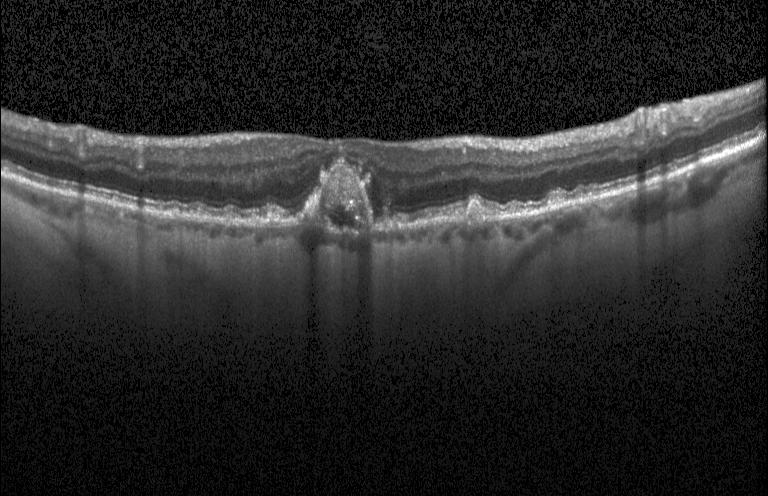

Fovea-centered · retinal OCT cross-section · instrument: Heidelberg Spectralis
Dx: choroidal neovascularization (CNV).